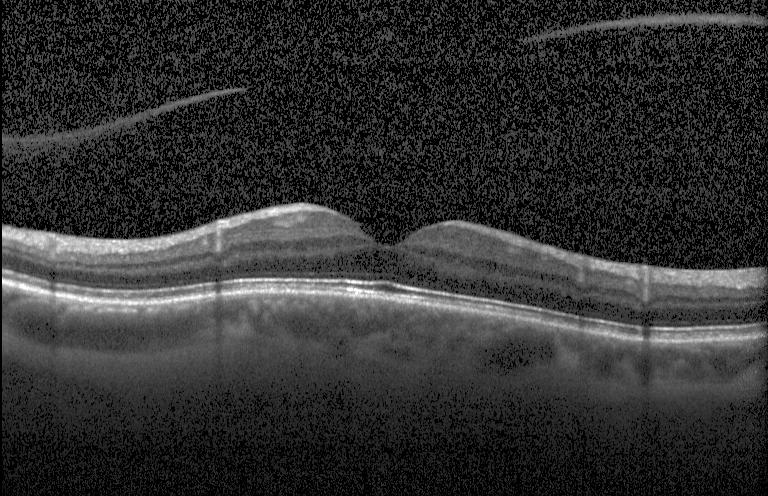

Diagnosis: no evidence of choroidal neovascularization, diabetic macular edema, or drusen.